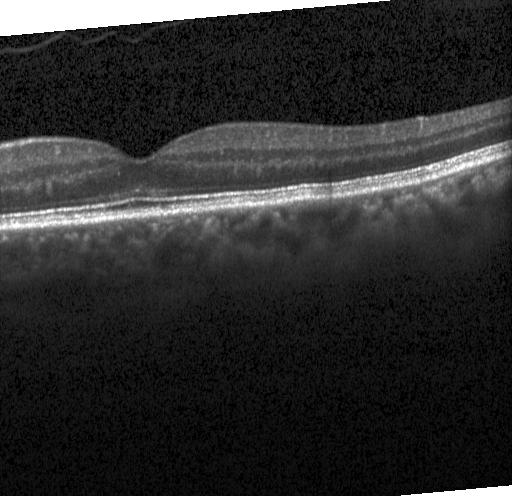 OCT line scan, SD-OCT. Finding: no evidence of choroidal neovascularization, diabetic macular edema, or drusen.